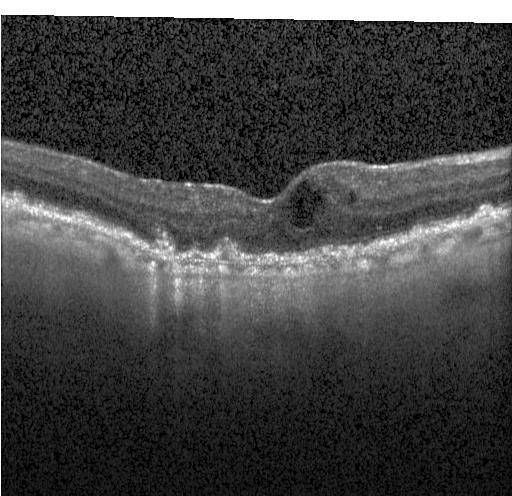 Spectral-domain OCT B-scan: a choroidal neovascular membrane.